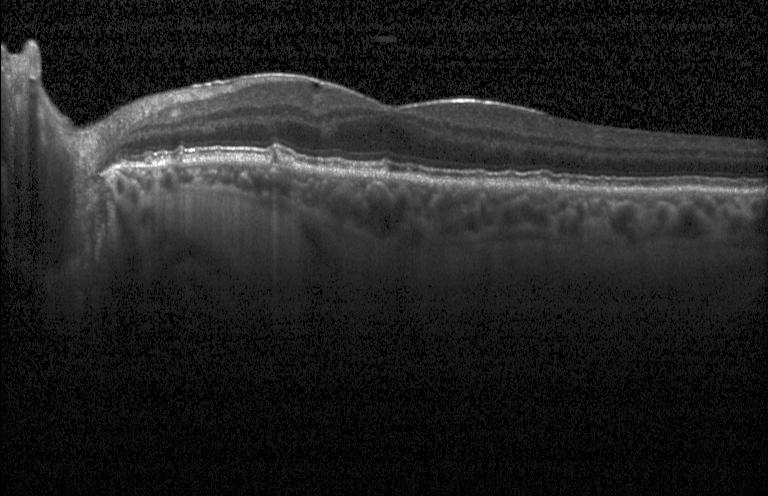 OCT finding: multiple drusen.